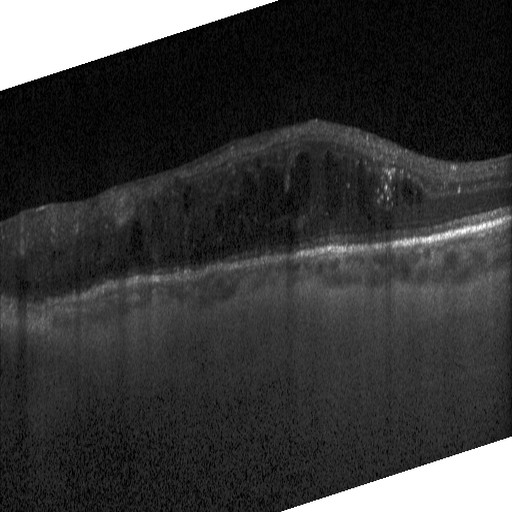

OCT B-scan showing DME.